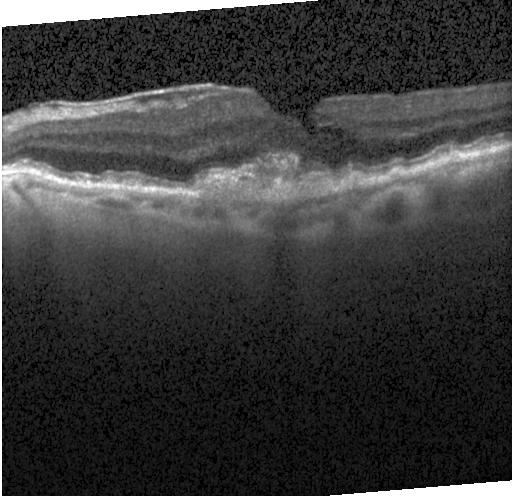
Dx: choroidal neovascularization.